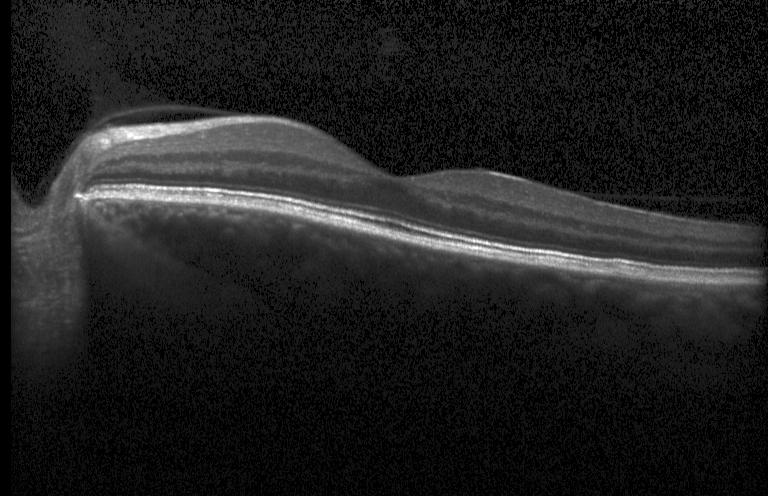
Fovea-centered. Optical coherence tomography B-scan. Spectral-domain OCT.
Finding: no choroidal neovascularization, diabetic macular edema, or drusen.